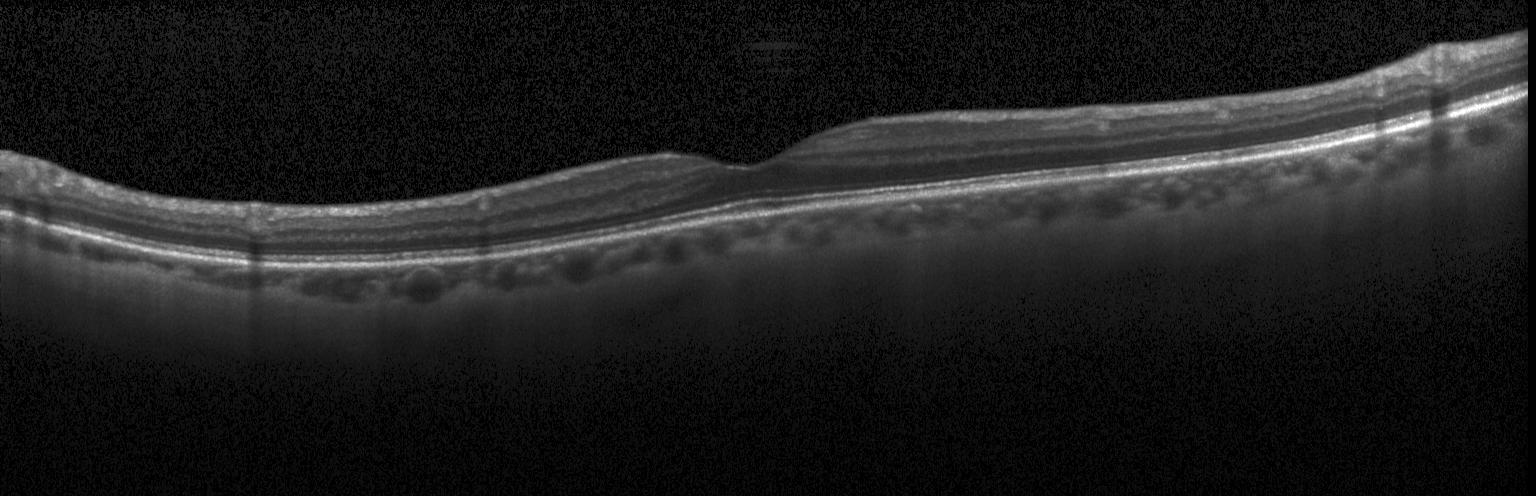

OCT B-scan — Diagnosis: neither CNV, DME, nor drusen.